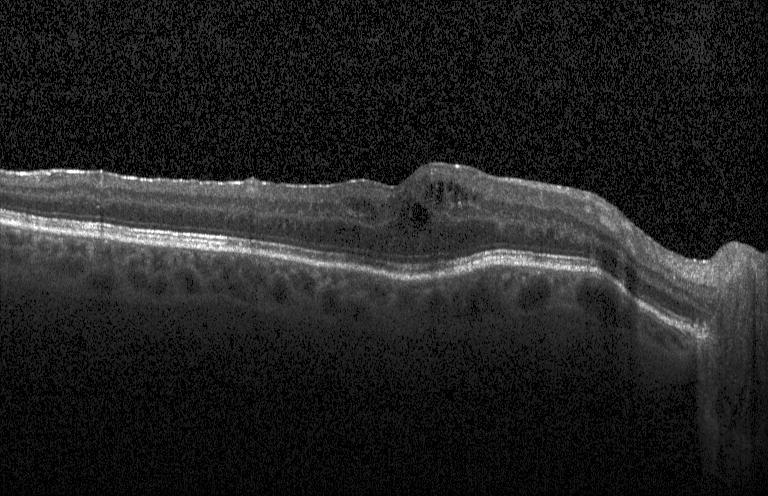

Spectral-domain optical coherence tomography, through the macula, OCT line scan, acquired on a Heidelberg Spectralis. This B-scan demonstrates DME.